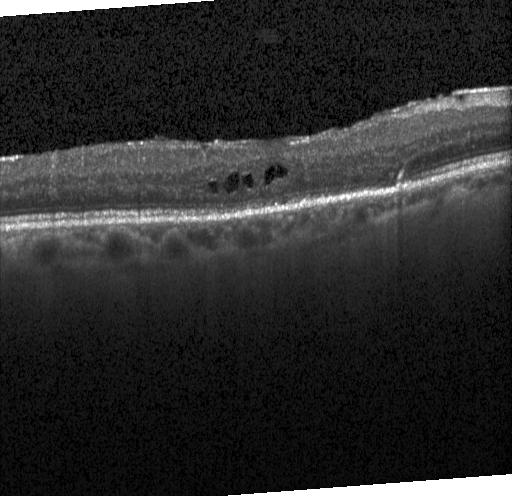 Macular OCT: DME.